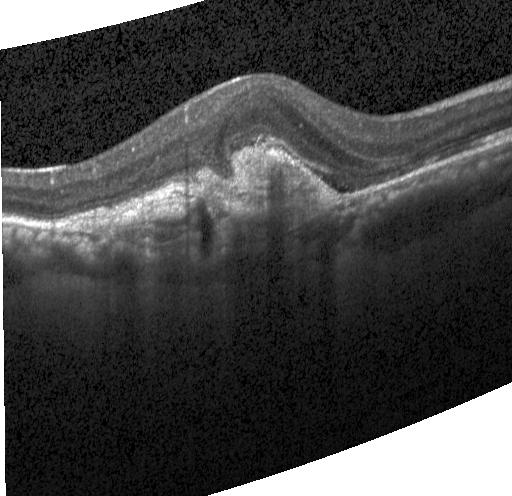

Diagnosis: a choroidal neovascular membrane.